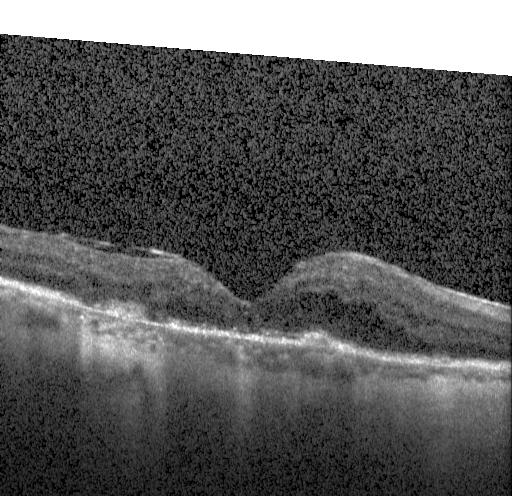 Macular scan; Heidelberg Spectralis OCT system; SD-OCT; retinal OCT cross-section
Dx: choroidal neovascularization.